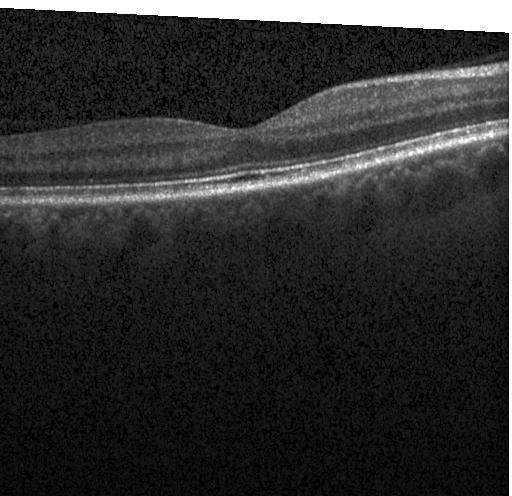
Finding: no choroidal neovascularization, diabetic macular edema, or drusen.